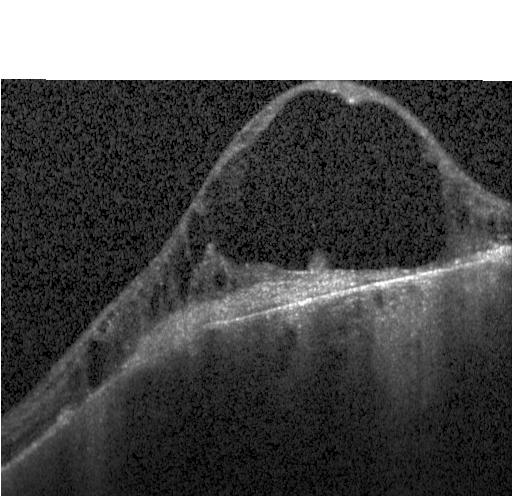
Spectral-domain OCT B-scan: a choroidal neovascular membrane.